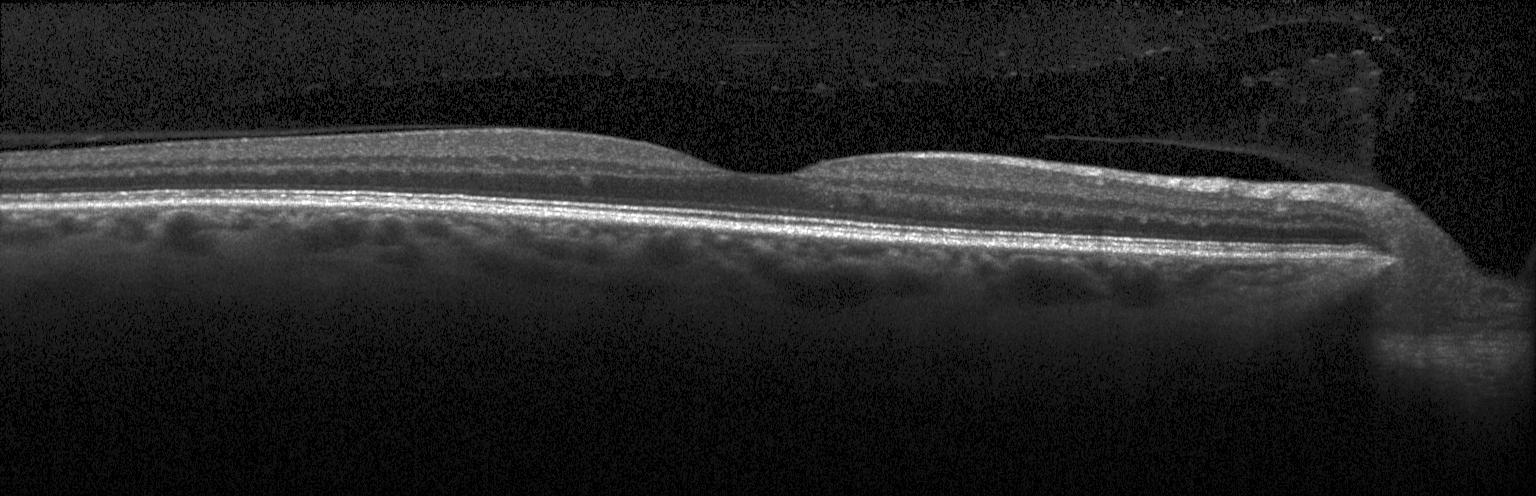 Macular scan · acquired on a Heidelberg Spectralis · OCT line scan · SD-OCT.
Diagnosis: no evidence of choroidal neovascularization, diabetic macular edema, or drusen.